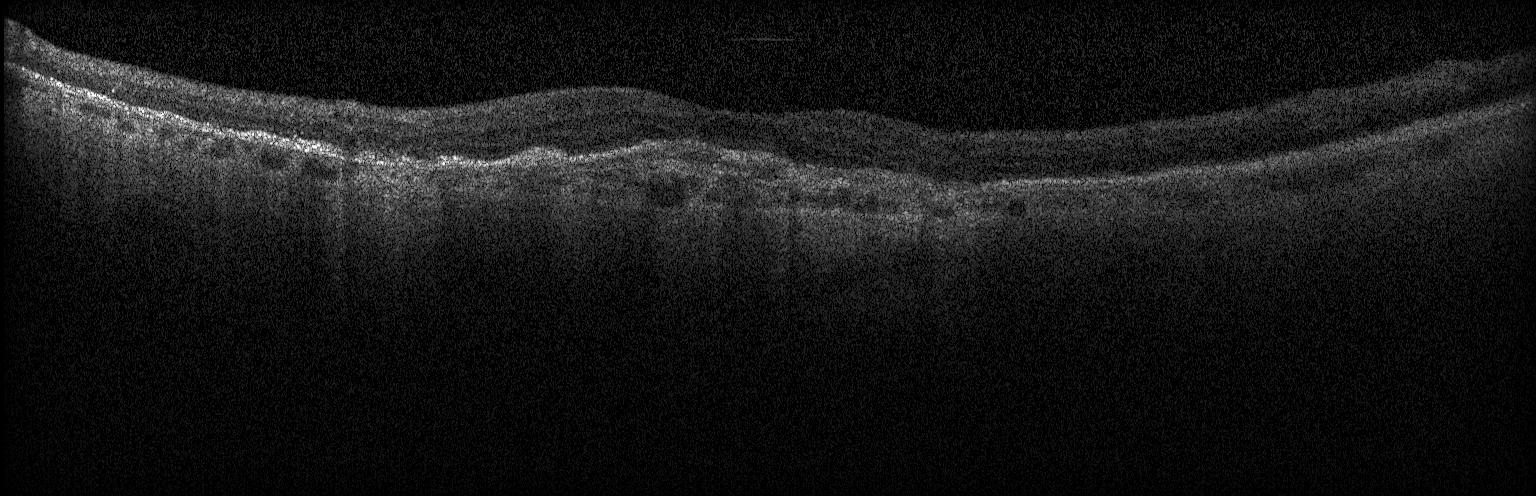
Retinal OCT cross-section showing choroidal neovascularization.